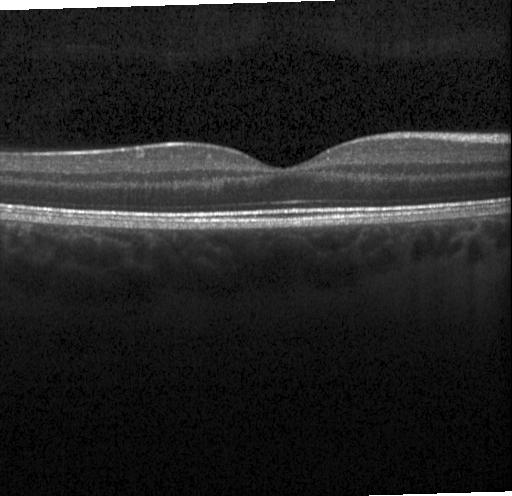 OCT line scan · spectral-domain optical coherence tomography · through the macula · instrument: Heidelberg Spectralis.
Diagnosis: neither choroidal neovascularization, diabetic macular edema, nor drusen.